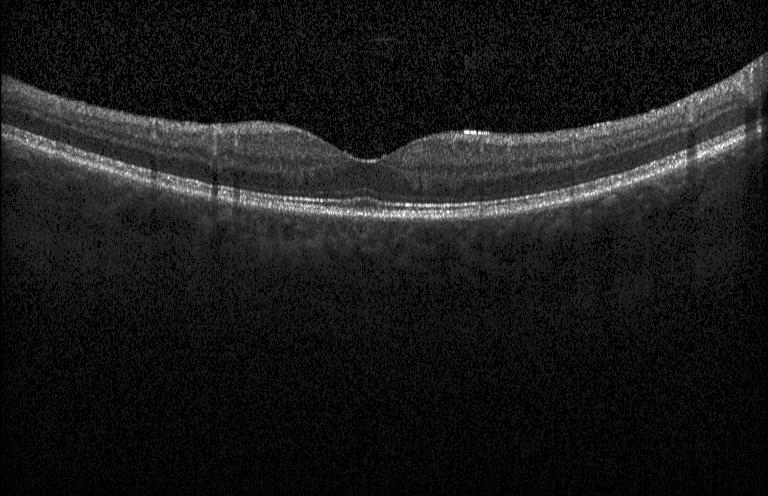
Spectral-domain optical coherence tomography. OCT line scan
Assessment: neither choroidal neovascularization, diabetic macular edema, nor drusen.